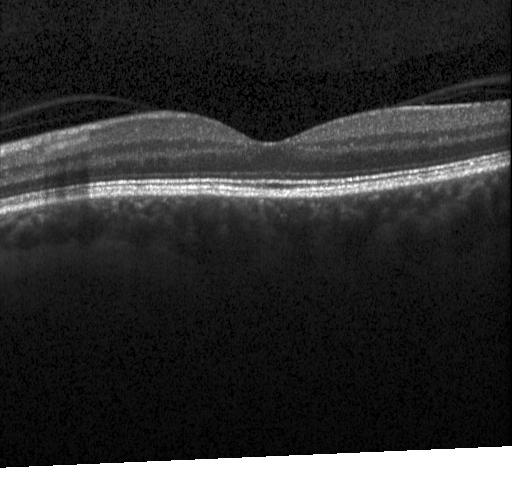

Retinal OCT cross-section
This B-scan demonstrates neither choroidal neovascularization, diabetic macular edema, nor drusen.